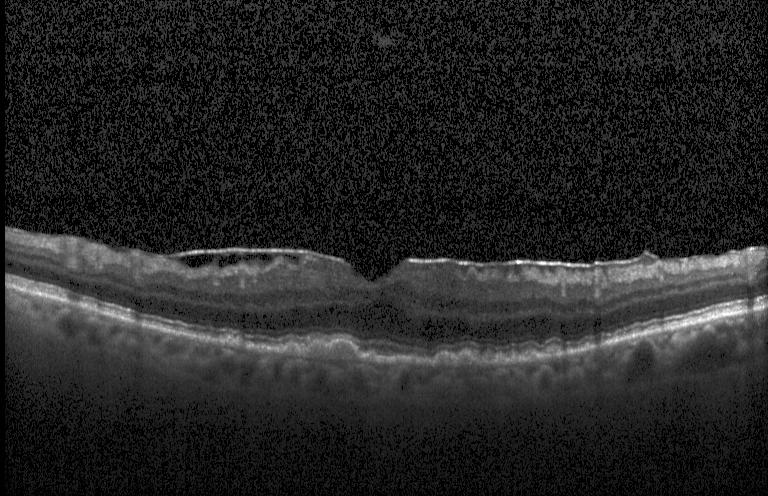

OCT scan showing sub-RPE drusenoid deposits.